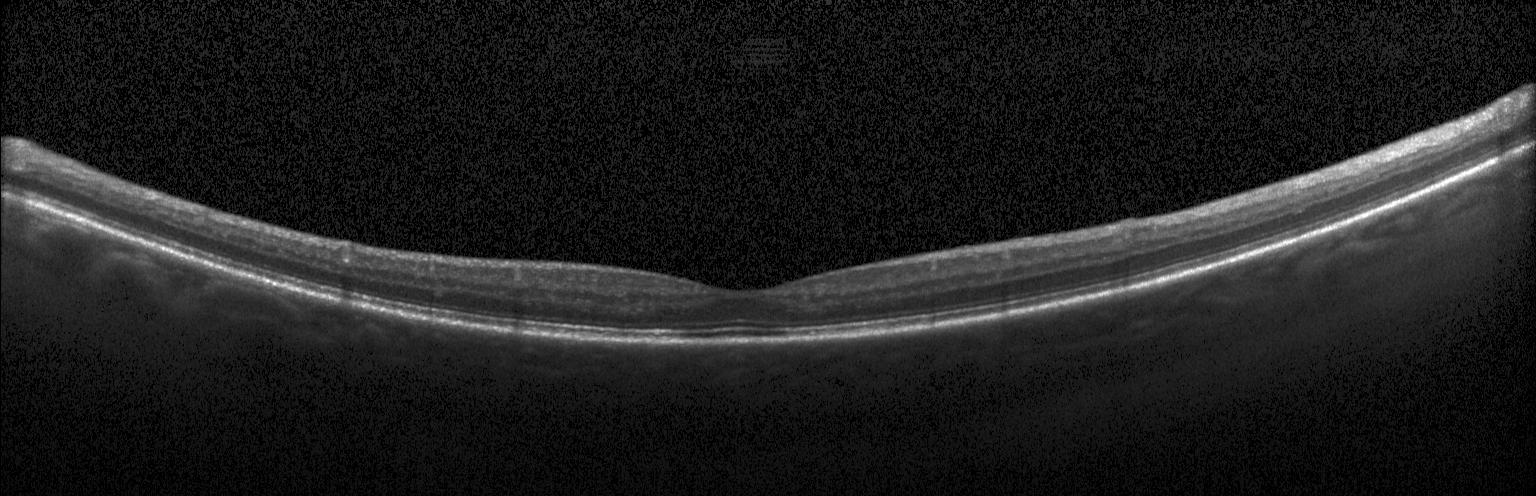
Impression: no evidence of choroidal neovascularization, diabetic macular edema, or drusen.